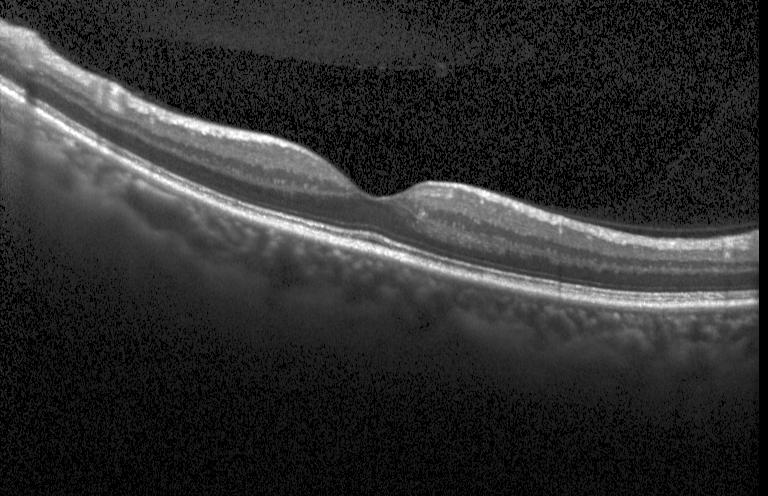

Heidelberg Spectralis OCT system, optical coherence tomography scan, through the macula, SD-OCT
Finding: no choroidal neovascularization, diabetic macular edema, or drusen.